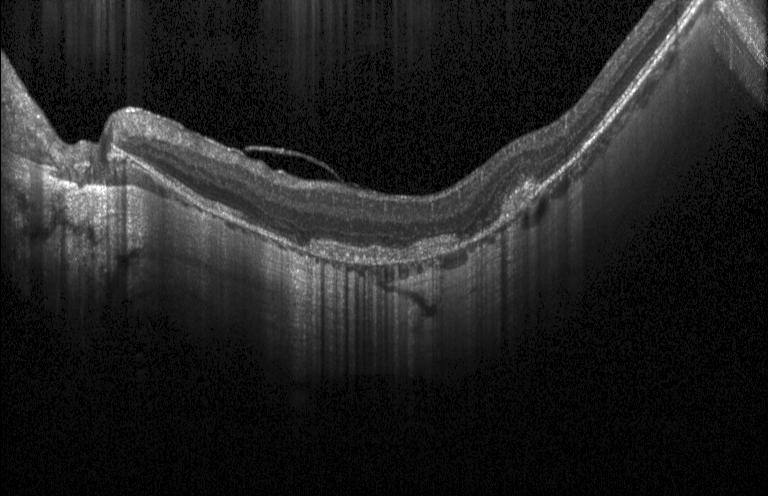 Centered on the fovea. Acquired on a Heidelberg Spectralis. OCT B-scan. Spectral-domain OCT — Assessment: a choroidal neovascular membrane.